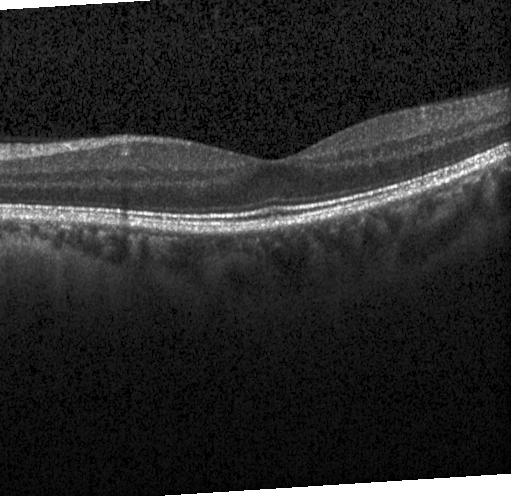 Assessment: no choroidal neovascularization, diabetic macular edema, or drusen.